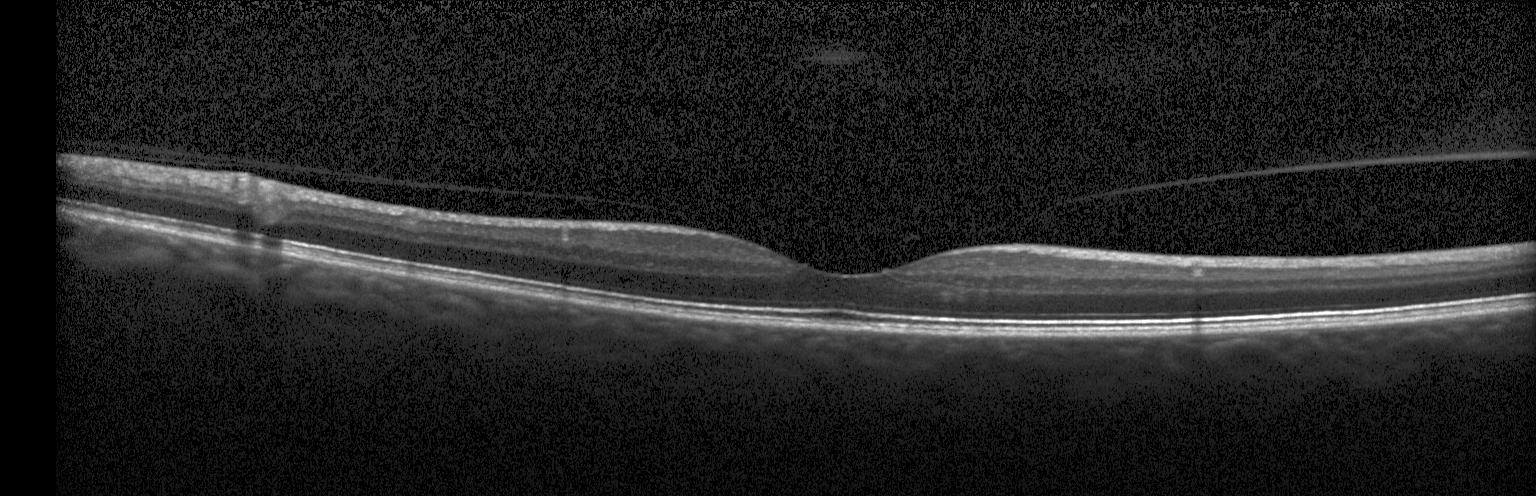 OCT B-scan — Macular OCT: neither choroidal neovascularization, diabetic macular edema, nor drusen.